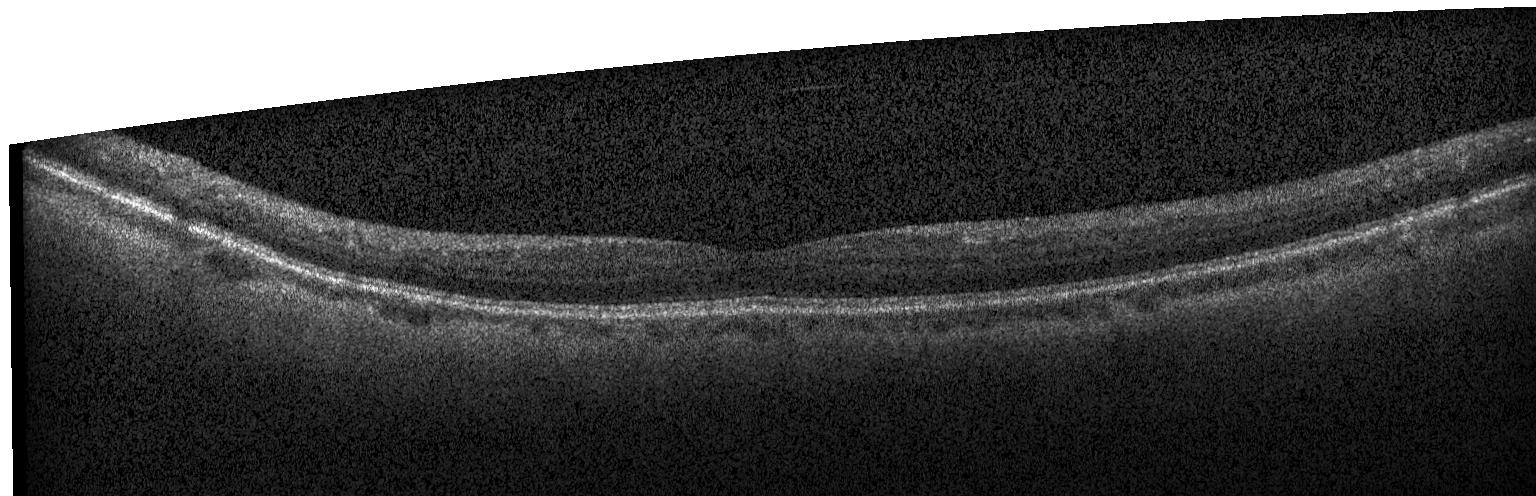
OCT line scan — The scan shows no choroidal neovascularization, diabetic macular edema, or drusen.